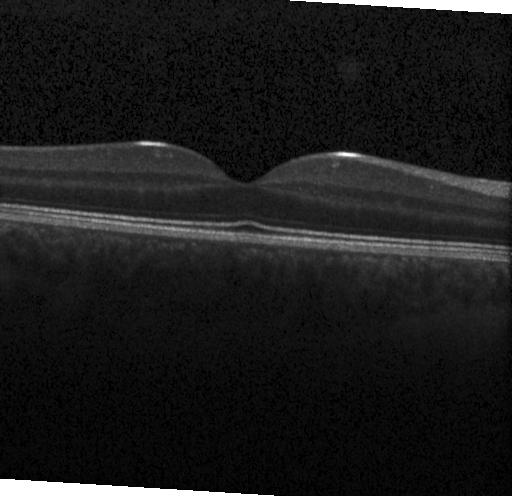
Retinal OCT cross-section showing no choroidal neovascularization, diabetic macular edema, or drusen.